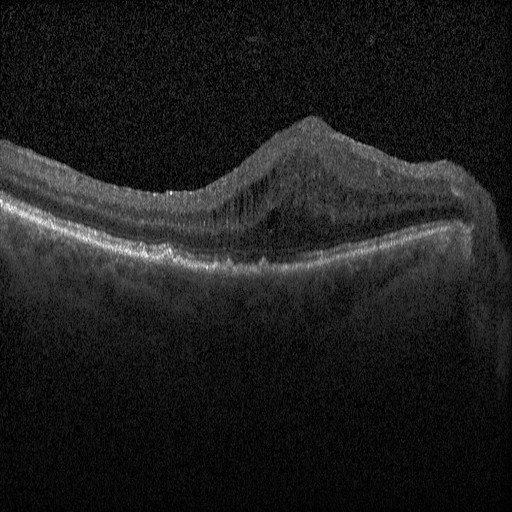

Optical coherence tomography B-scan
Finding: DME.